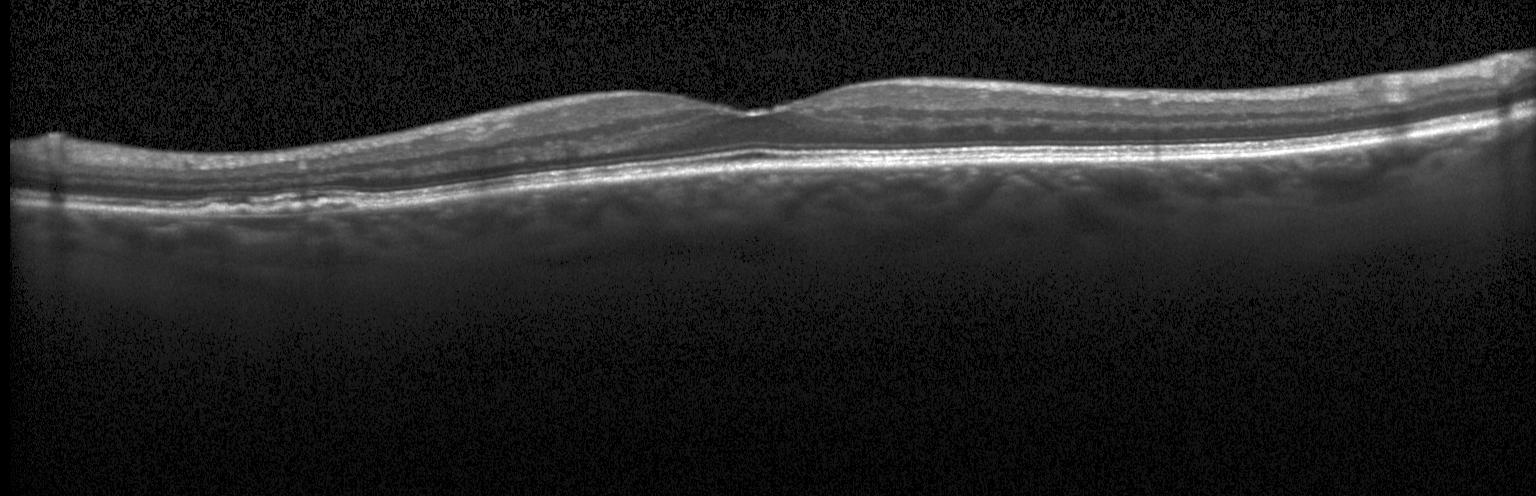

OCT line scan; instrument: Heidelberg Spectralis. Finding: a choroidal neovascular membrane.